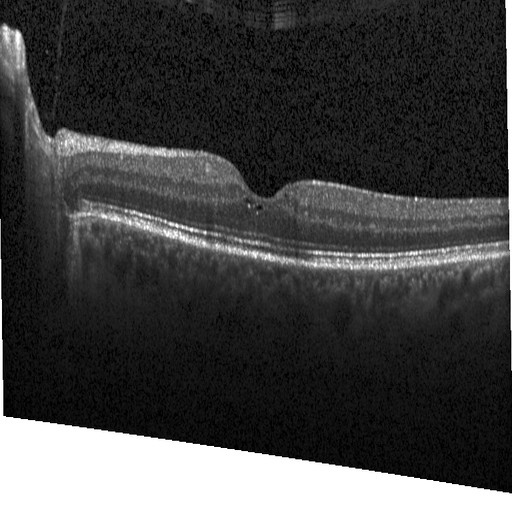 OCT B-scan showing diabetic macular edema (DME).